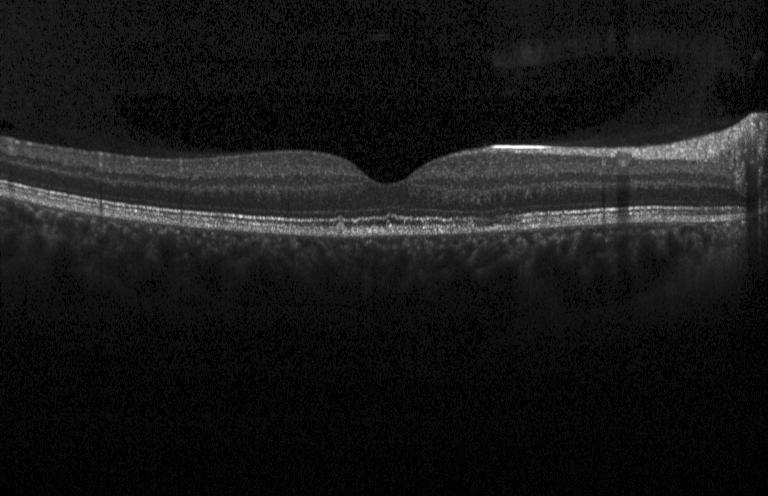

Through the macula. OCT line scan — OCT finding: multiple drusen.